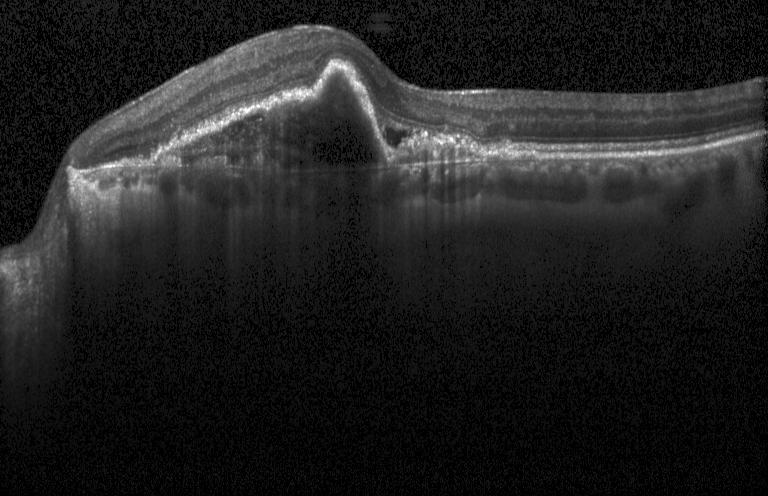

Macular OCT: a choroidal neovascular membrane.